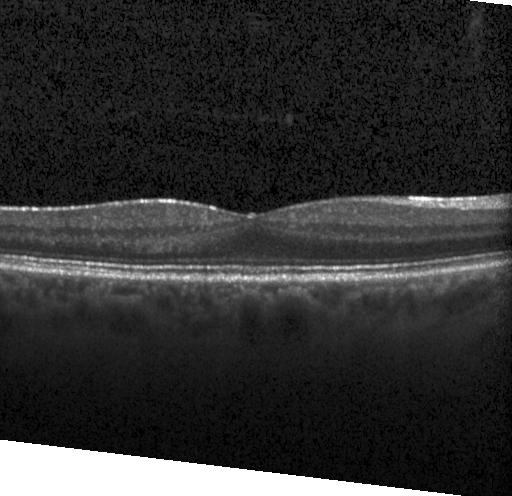

Macular OCT: no evidence of choroidal neovascularization, diabetic macular edema, or drusen.